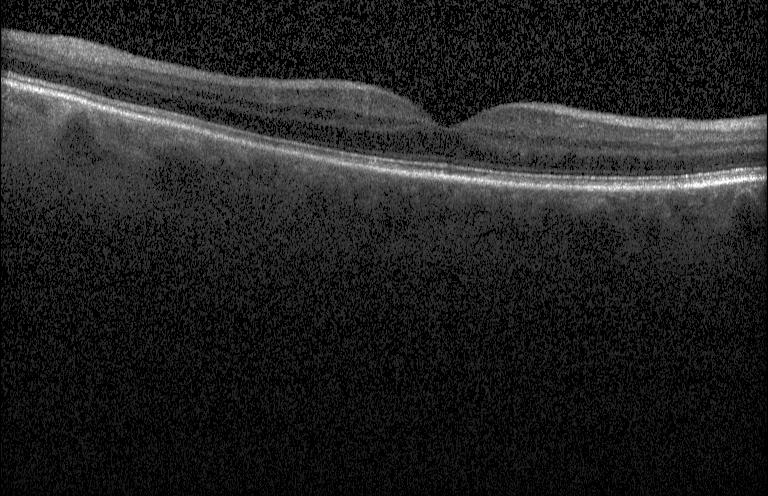

Retinal OCT cross-section — Diagnosis: no choroidal neovascularization, no diabetic macular edema, and no drusen.